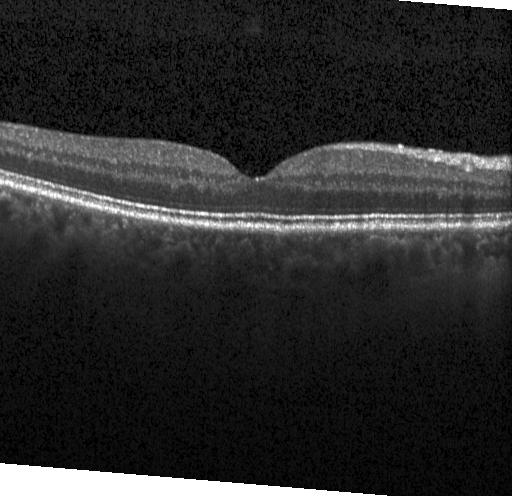

Horizontal scan through the fovea, optical coherence tomography scan
Finding: no choroidal neovascularization, diabetic macular edema, or drusen.